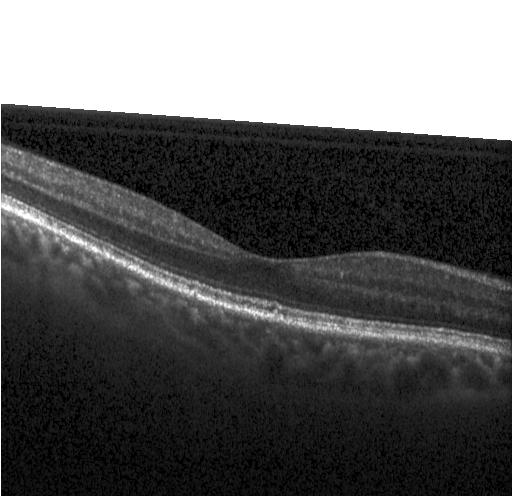

Diagnosis: no evidence of CNV, DME, or drusen.